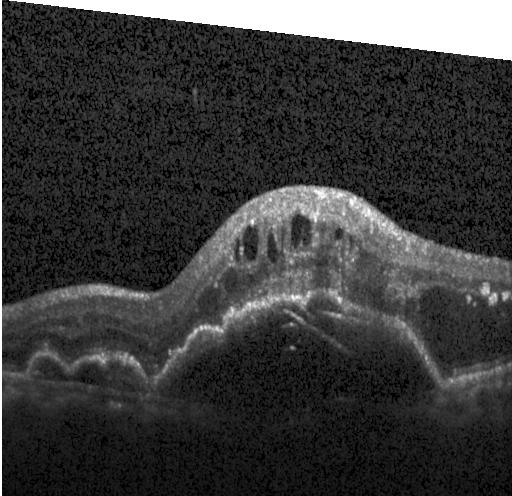 Fovea-centered · spectral-domain OCT · Heidelberg Spectralis · retinal OCT cross-section. Diagnosis: a choroidal neovascular membrane.